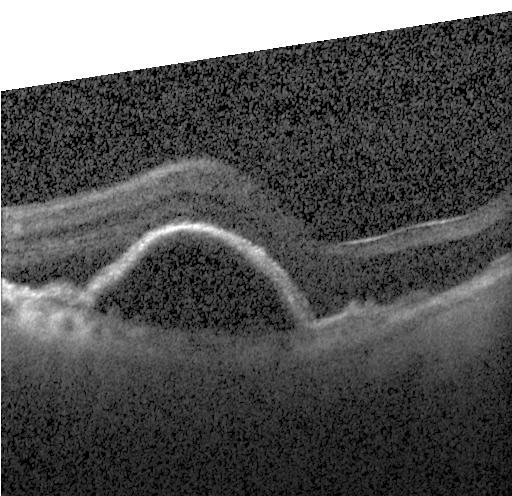

Assessment: a choroidal neovascular membrane.